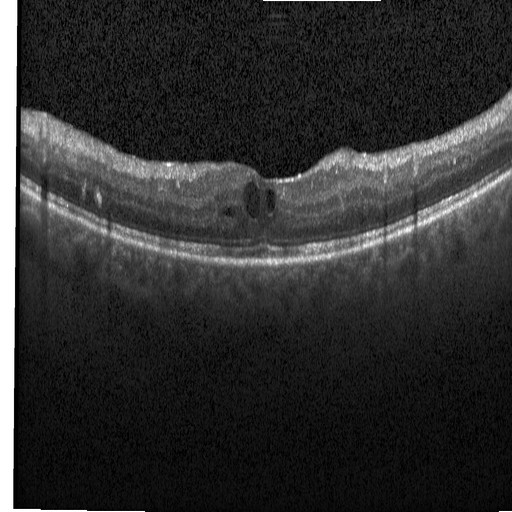

Finding: diabetic macular edema.